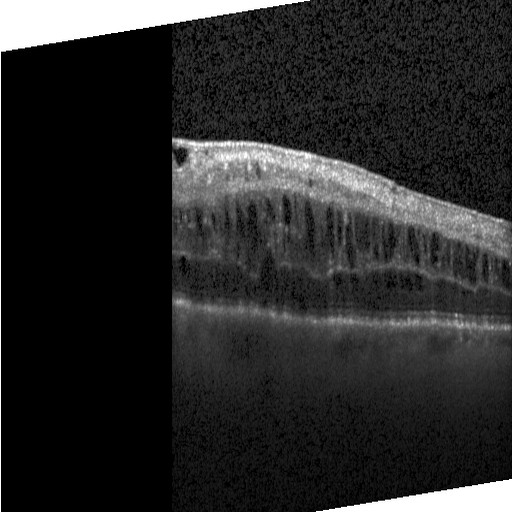 Diabetic macular edema.